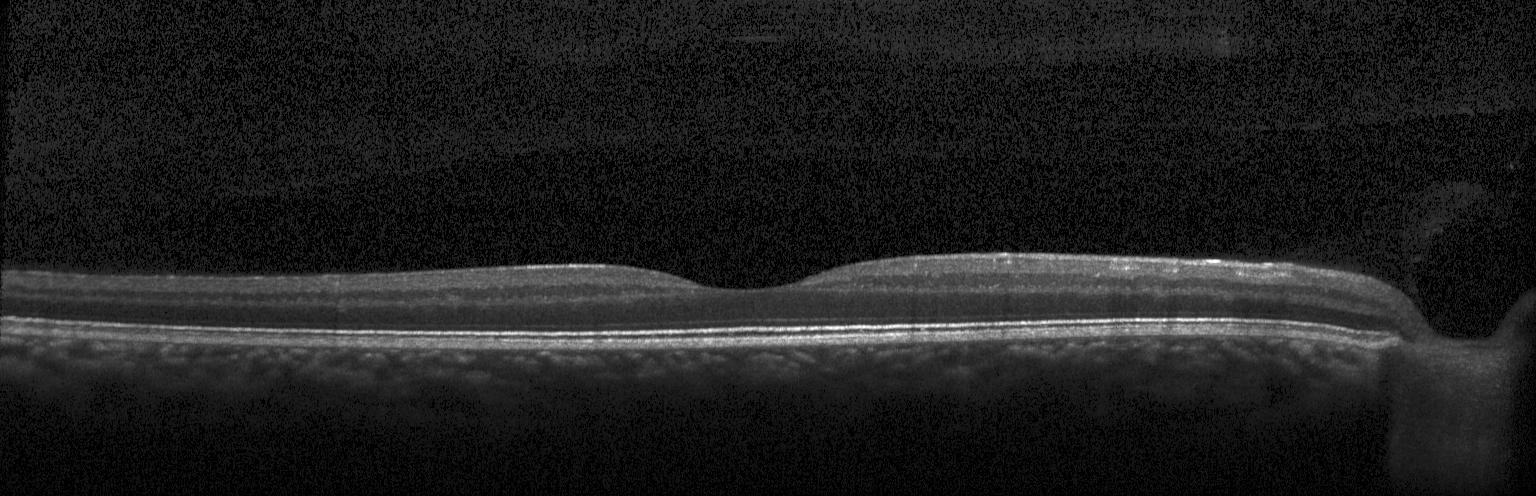

Macular scan, instrument: Heidelberg Spectralis, SD-OCT, OCT line scan — Diagnosis: no choroidal neovascularization, no diabetic macular edema, and no drusen.